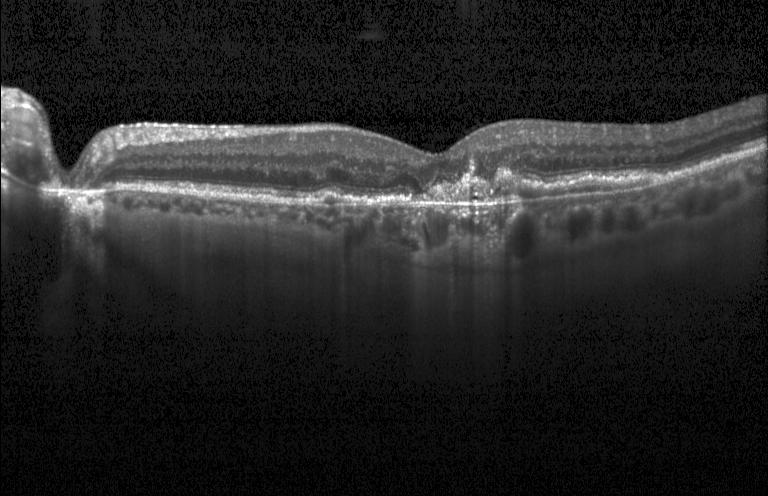

OCT scan showing a choroidal neovascular membrane.